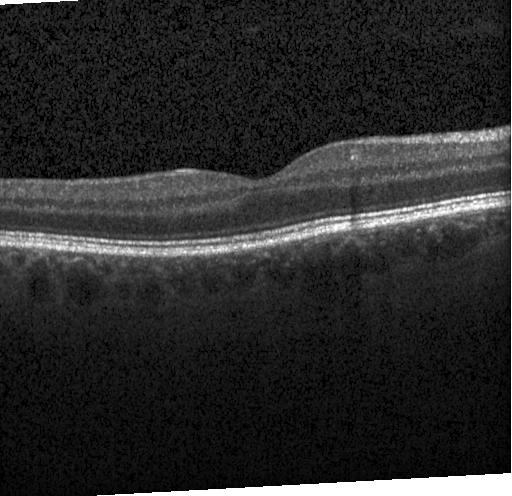 Finding: neither choroidal neovascularization, diabetic macular edema, nor drusen.